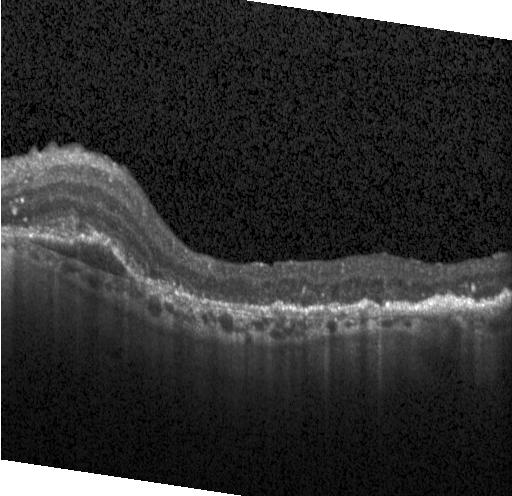

Finding: choroidal neovascularization (CNV).